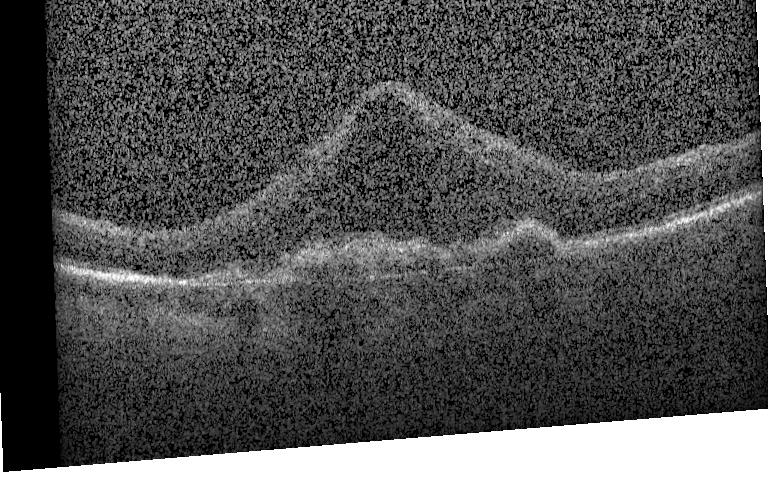
OCT line scan · Heidelberg Spectralis OCT system.
Dx: a choroidal neovascular membrane.